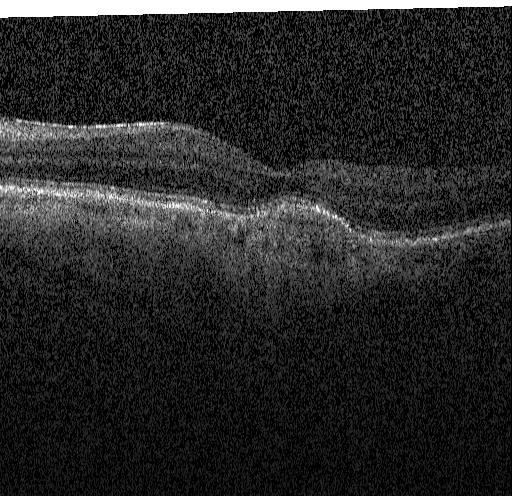

Diagnosis: choroidal neovascularization (CNV).